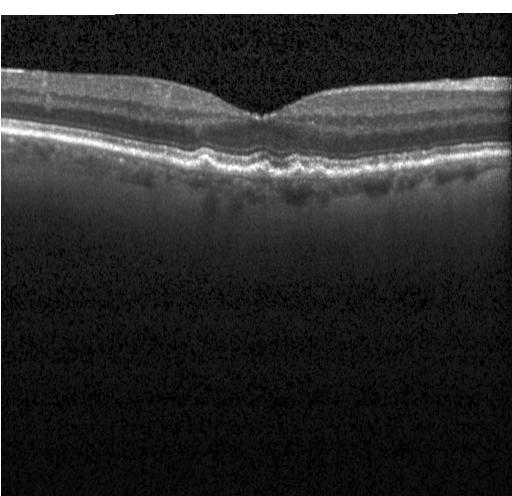

Optical coherence tomography scan; macular scan; Heidelberg Spectralis OCT system. Finding: sub-RPE drusenoid deposits.